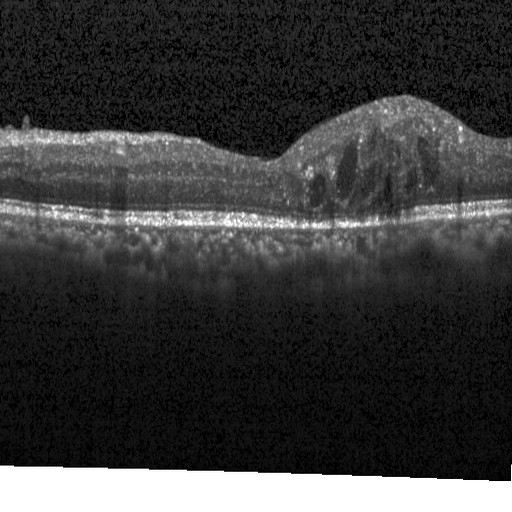

Acquired on a Heidelberg Spectralis. Spectral-domain OCT. Horizontal scan through the fovea. Optical coherence tomography scan. Impression: diabetic macular edema (DME).